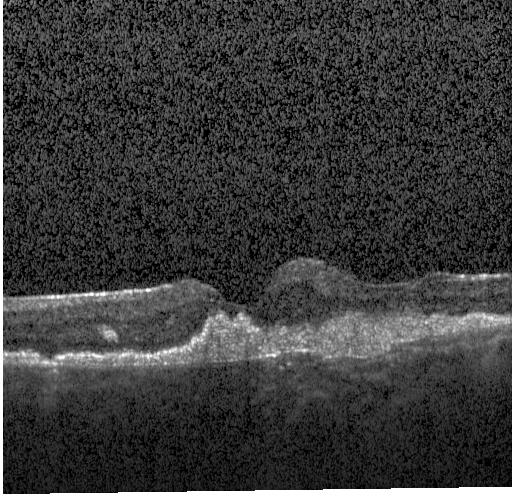

SD-OCT, through the macula, acquired on a Heidelberg Spectralis, OCT line scan. Diagnosis: choroidal neovascularization.